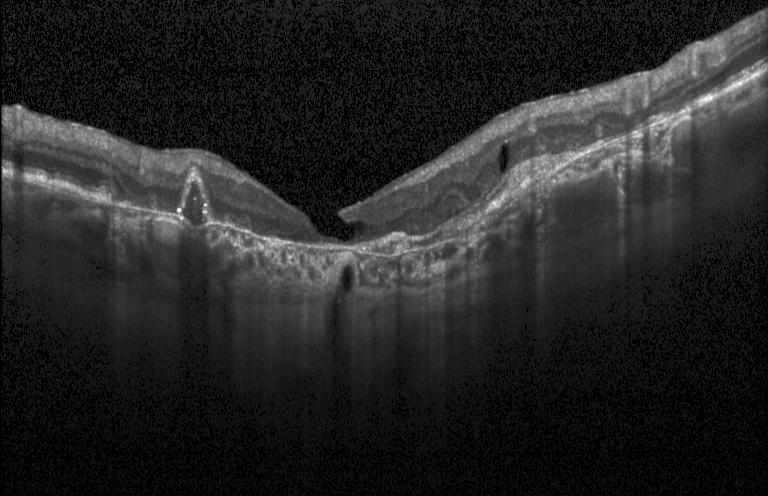 OCT line scan
The scan shows CNV.